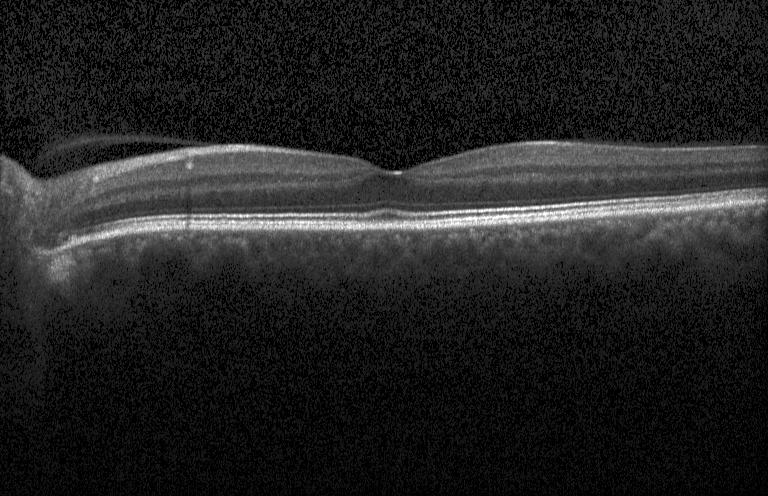 OCT finding: no choroidal neovascularization, diabetic macular edema, or drusen.